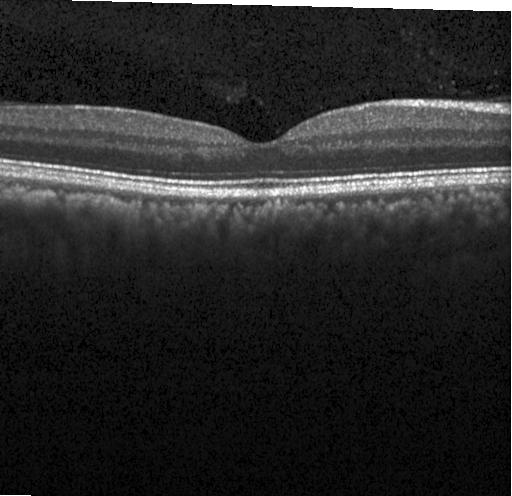

Optical coherence tomography B-scan. Instrument: Heidelberg Spectralis. Horizontal scan through the fovea.
Macular OCT: no evidence of CNV, DME, or drusen.